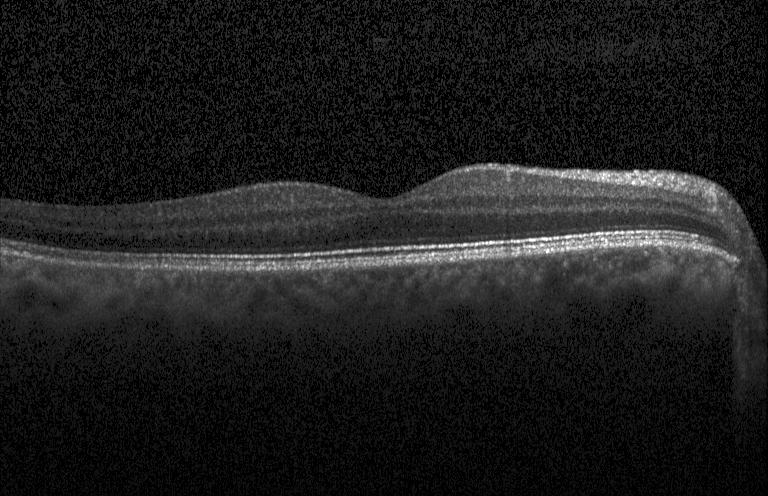
Horizontal scan through the fovea; OCT B-scan; instrument: Heidelberg Spectralis; spectral-domain optical coherence tomography — Assessment: no evidence of choroidal neovascularization, diabetic macular edema, or drusen.